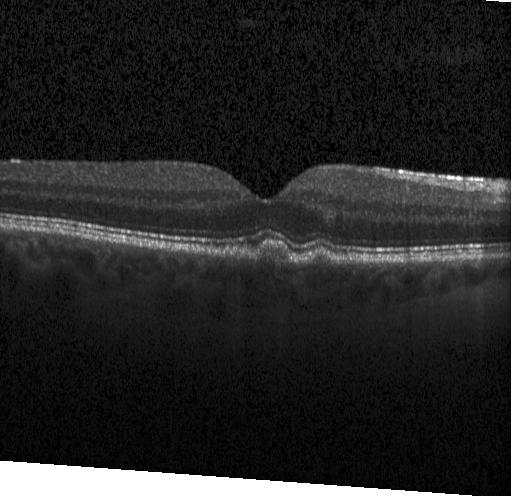
Diagnosis: sub-RPE drusenoid deposits.